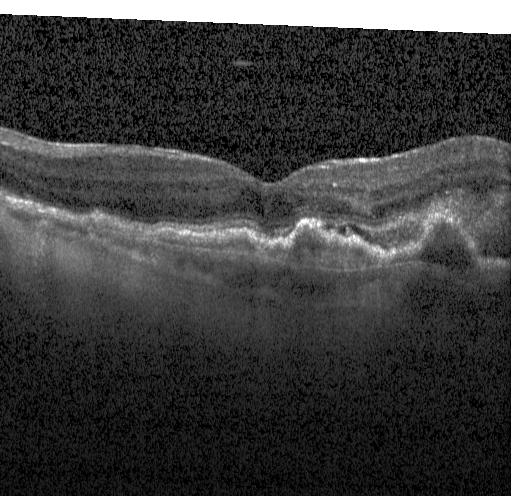
Dx: a choroidal neovascular membrane.